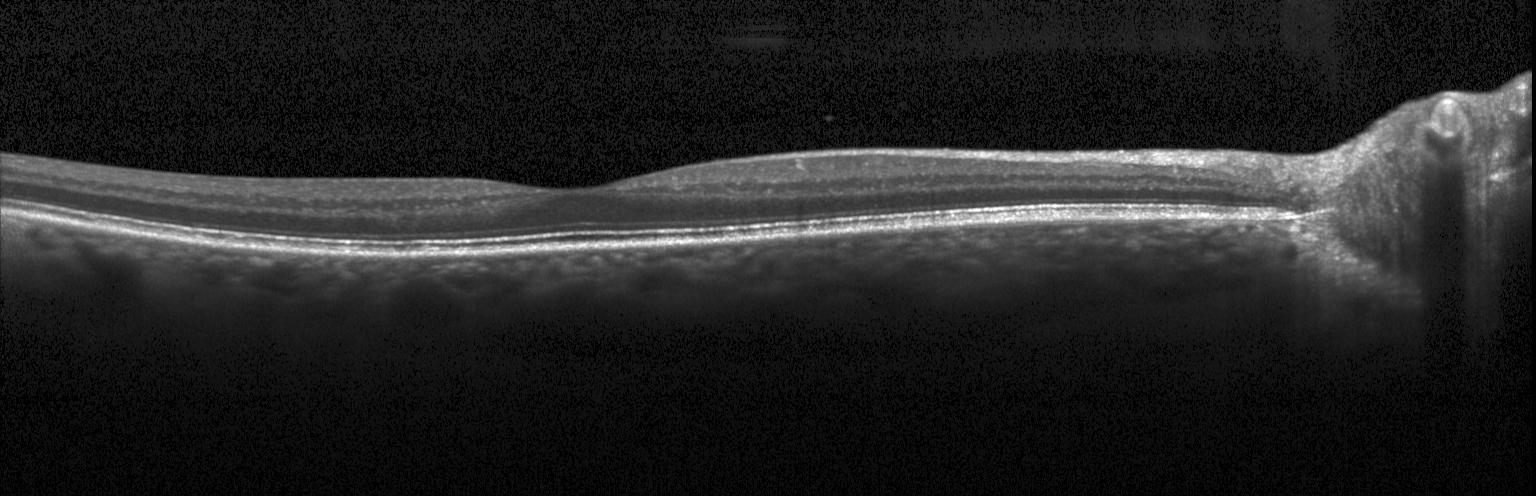 Instrument: Heidelberg Spectralis. OCT line scan — Assessment: neither choroidal neovascularization, diabetic macular edema, nor drusen.